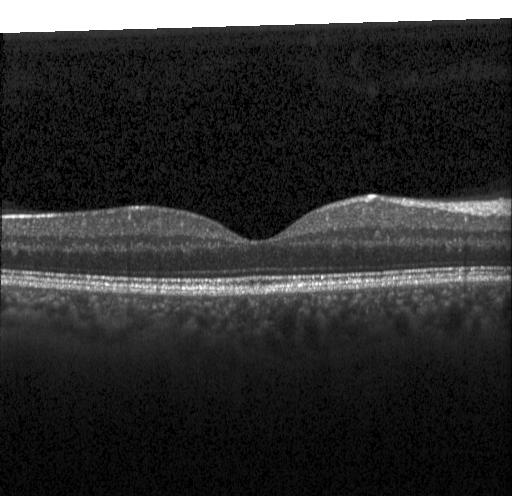

OCT finding: no choroidal neovascularization, no diabetic macular edema, and no drusen.